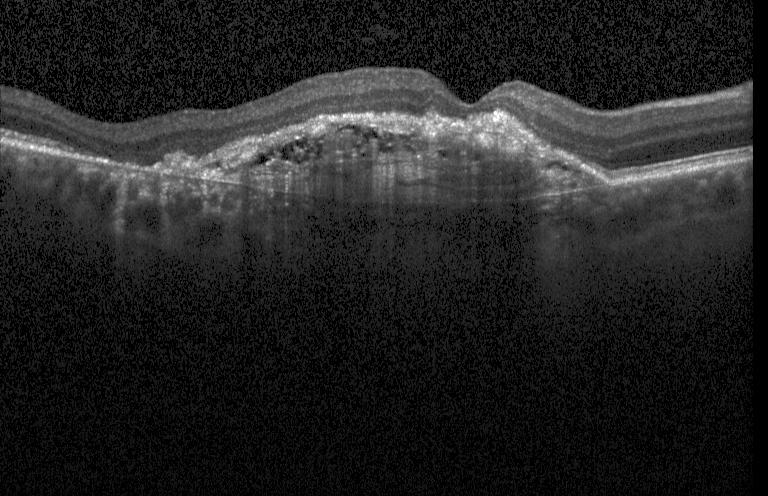
This B-scan demonstrates a choroidal neovascular membrane.